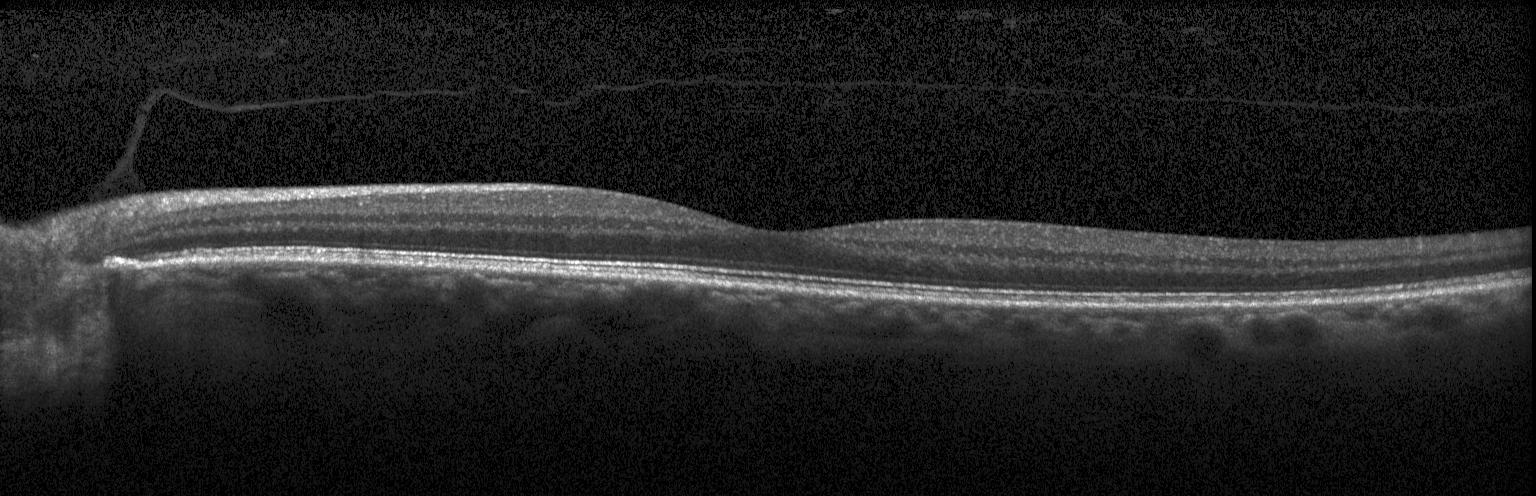 Finding: no CNV, no DME, and no drusen.